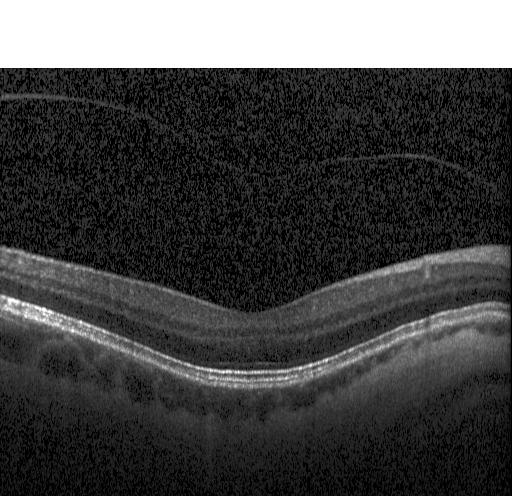

Retinal OCT B-scan.
Impression: no choroidal neovascularization, diabetic macular edema, or drusen.